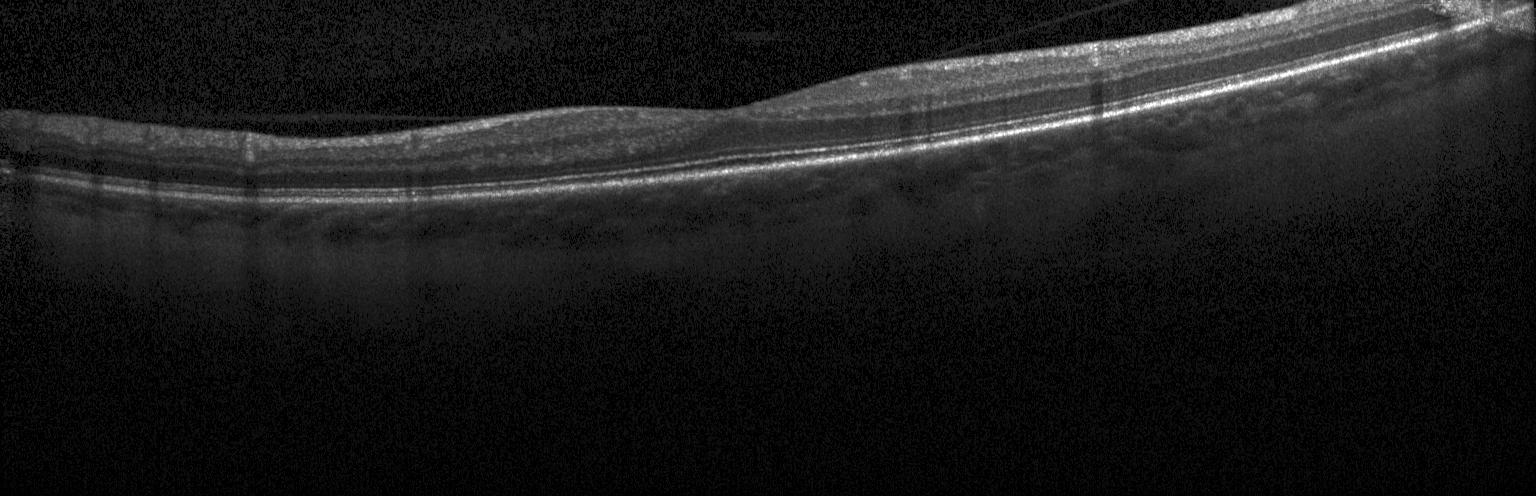
This B-scan demonstrates neither choroidal neovascularization, diabetic macular edema, nor drusen.